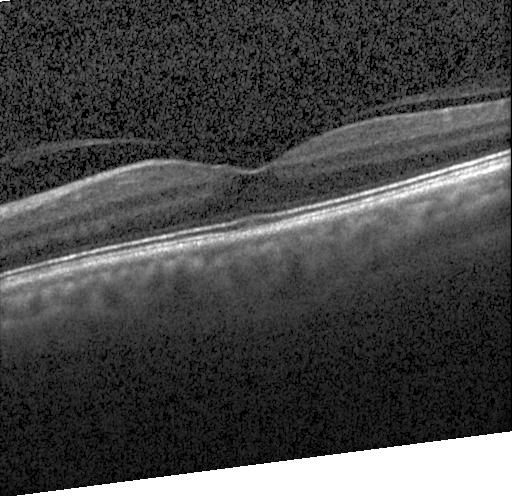
Heidelberg Spectralis OCT system; macular scan; SD-OCT; OCT line scan — This B-scan demonstrates no evidence of choroidal neovascularization, diabetic macular edema, or drusen.